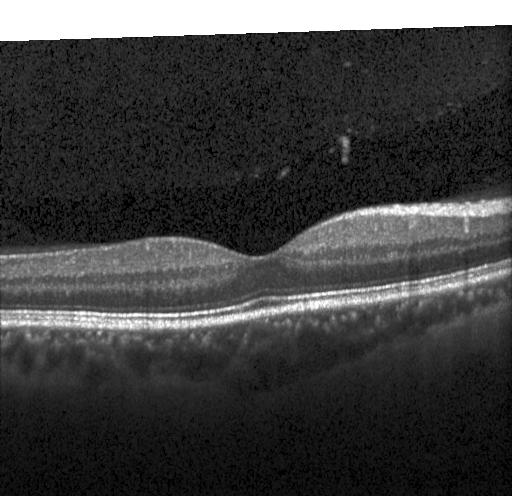
Heidelberg Spectralis OCT system. Spectral-domain optical coherence tomography. Through the macula. Optical coherence tomography B-scan. The scan shows neither CNV, DME, nor drusen.